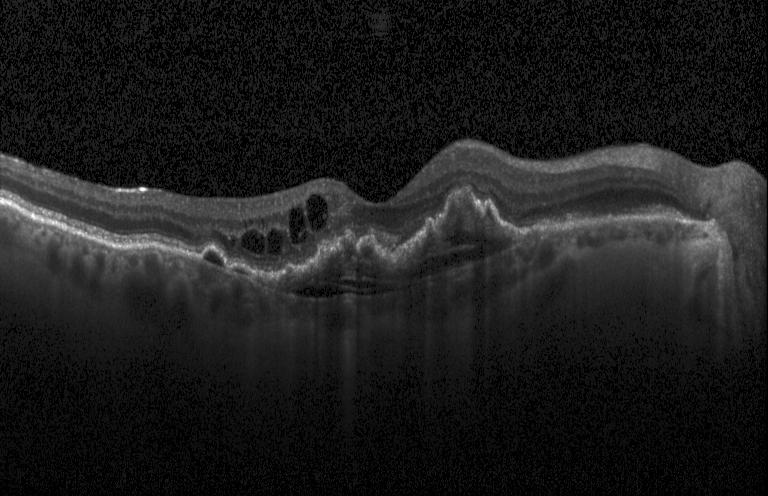 Retinal OCT B-scan; macular scan; spectral-domain optical coherence tomography. Choroidal neovascularization (CNV).